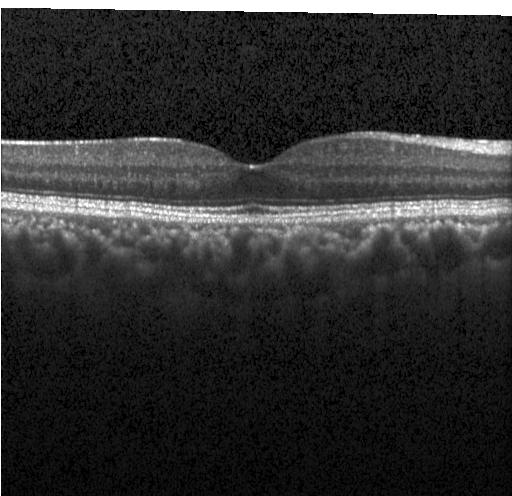

Dx: no choroidal neovascularization, diabetic macular edema, or drusen.